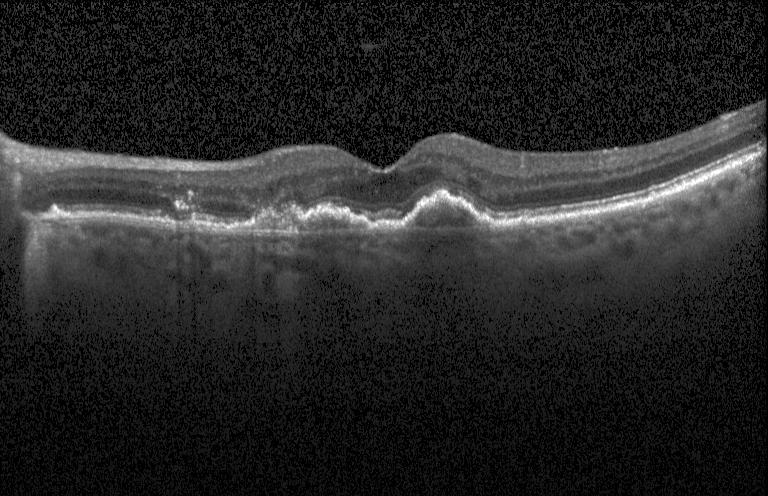 Diagnosis: a choroidal neovascular membrane.